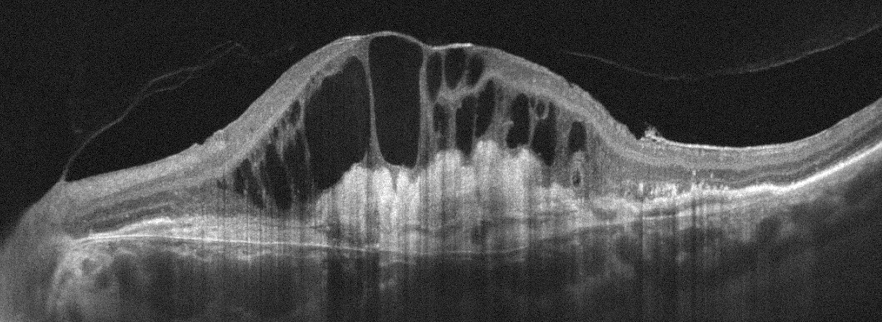
Optovue Avanti RTVue XR; through the macula; oculus sinister; OCT B-scan.
Impression: age-related macular degeneration.